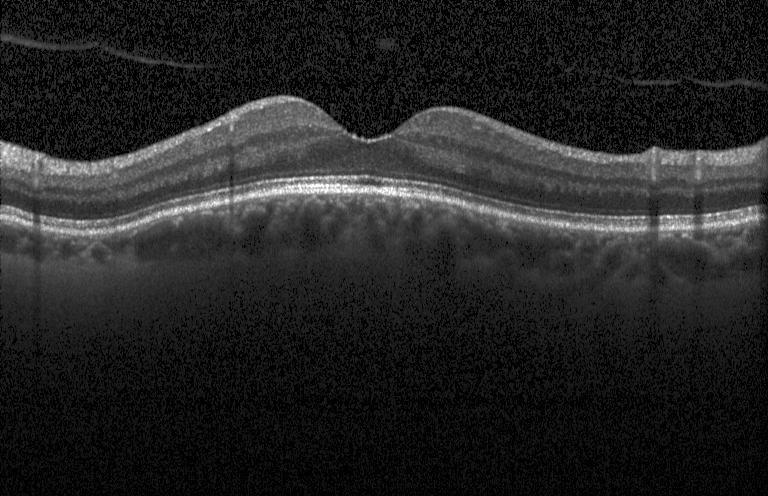

Spectral-domain OCT. OCT B-scan. Heidelberg Spectralis OCT system. Macular scan — This B-scan demonstrates no evidence of choroidal neovascularization, diabetic macular edema, or drusen.